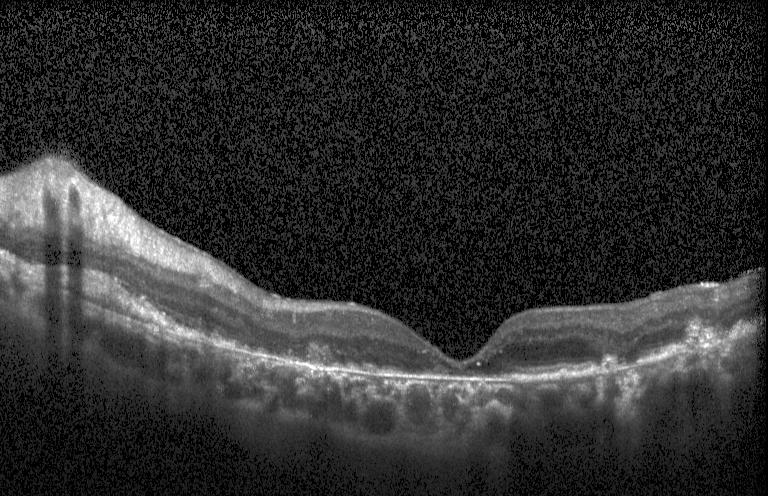 Retinal OCT B-scan · fovea-centered — Impression: a choroidal neovascular membrane.